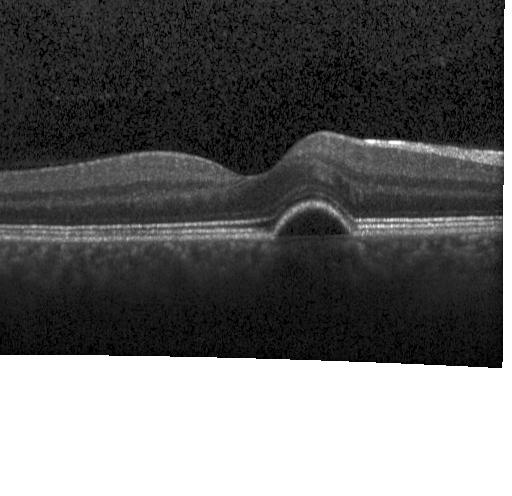
Instrument: Heidelberg Spectralis, optical coherence tomography B-scan, spectral-domain OCT, horizontal scan through the fovea. The scan shows choroidal neovascularization (CNV).